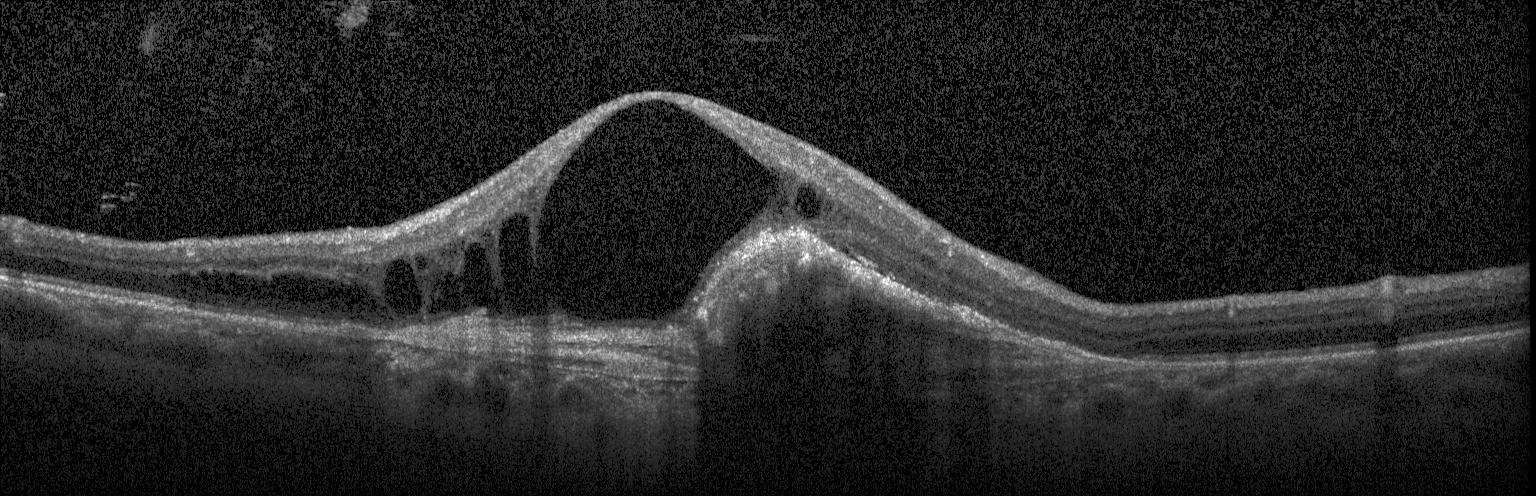 Retinal OCT cross-section — Impression: a choroidal neovascular membrane.